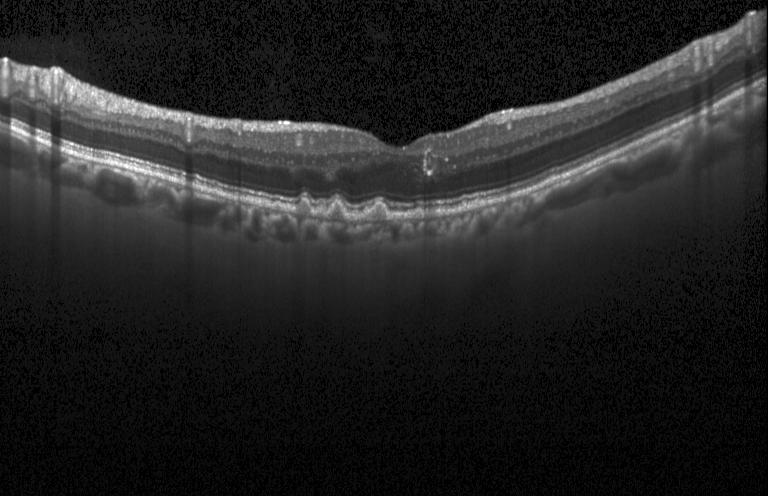 Retinal OCT B-scan; acquired on a Heidelberg Spectralis; spectral-domain optical coherence tomography. Macular OCT: multiple drusen.